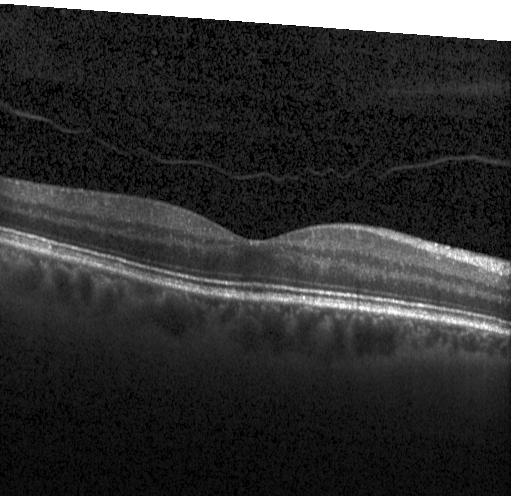

Retinal OCT cross-section · macular scan
Finding: no evidence of CNV, DME, or drusen.